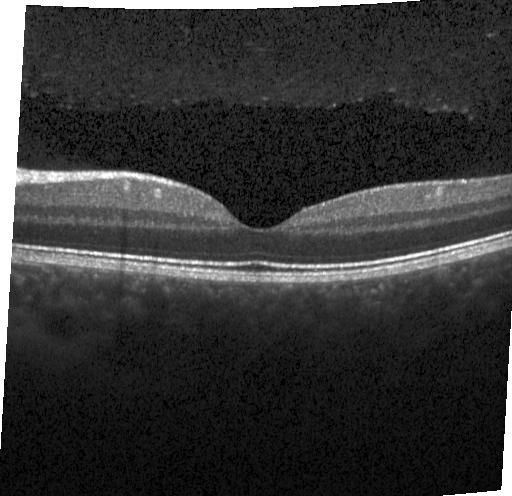 OCT finding: no CNV, no DME, and no drusen.